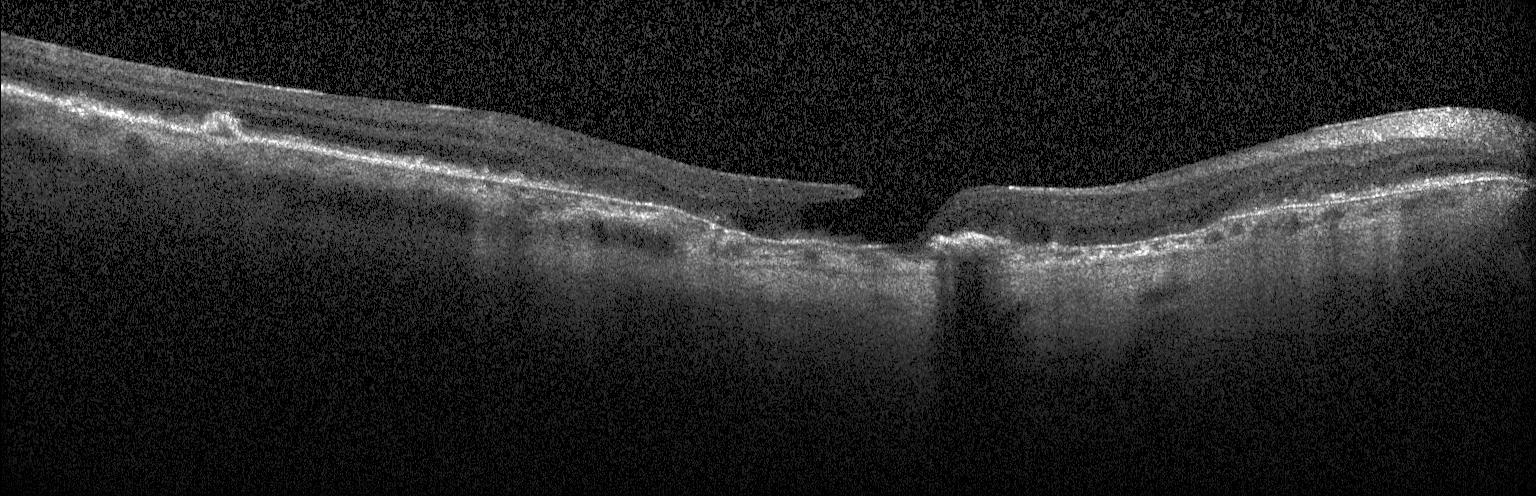
Finding: choroidal neovascularization.